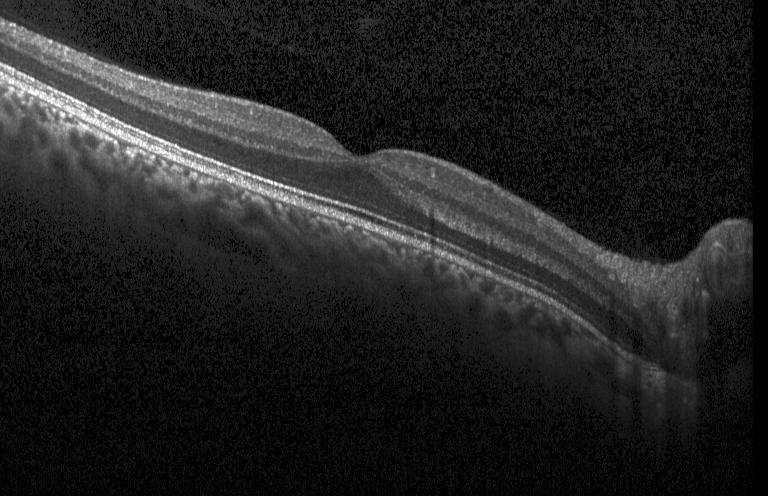

OCT line scan. Impression: no choroidal neovascularization, diabetic macular edema, or drusen.